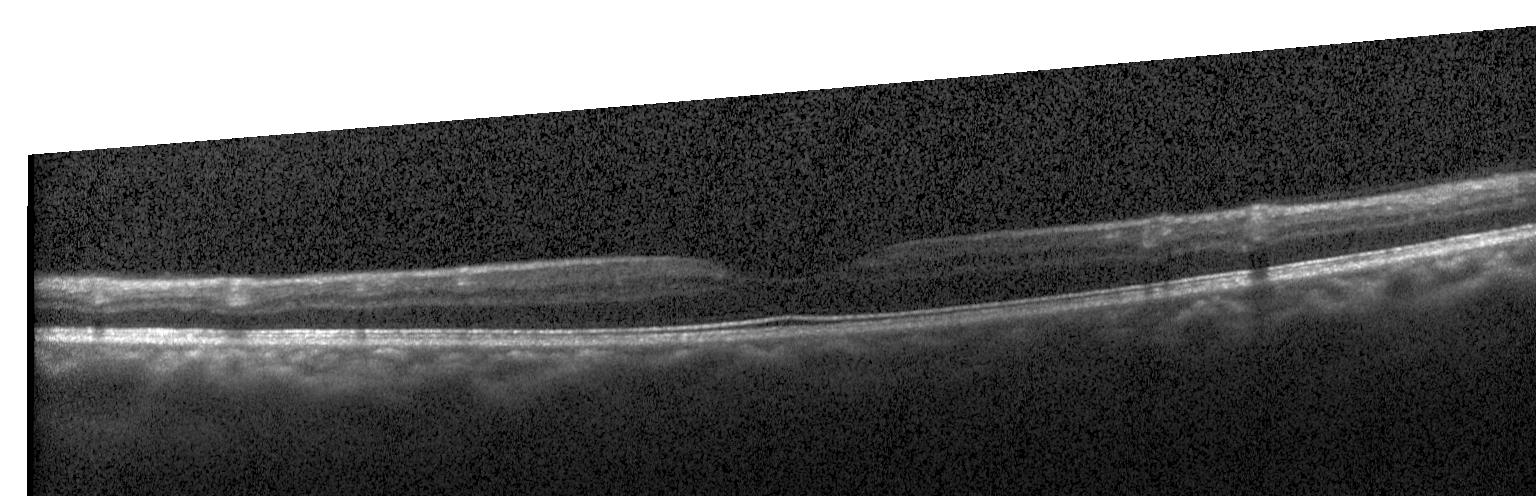

Spectral-domain OCT · macular scan · OCT line scan · acquired on a Heidelberg Spectralis.
Diagnosis: neither choroidal neovascularization, diabetic macular edema, nor drusen.